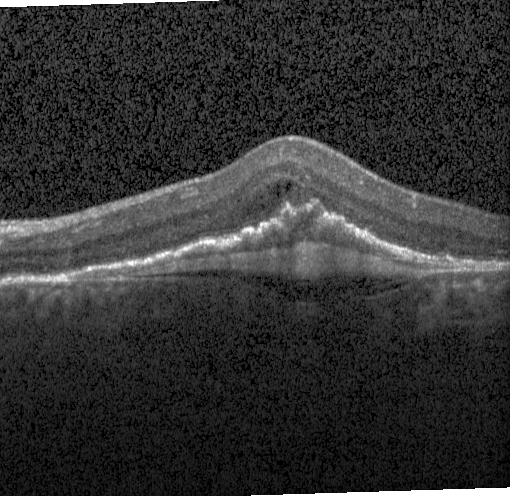

Optical coherence tomography scan; acquired on a Heidelberg Spectralis; centered on the fovea; SD-OCT.
Assessment: a choroidal neovascular membrane.